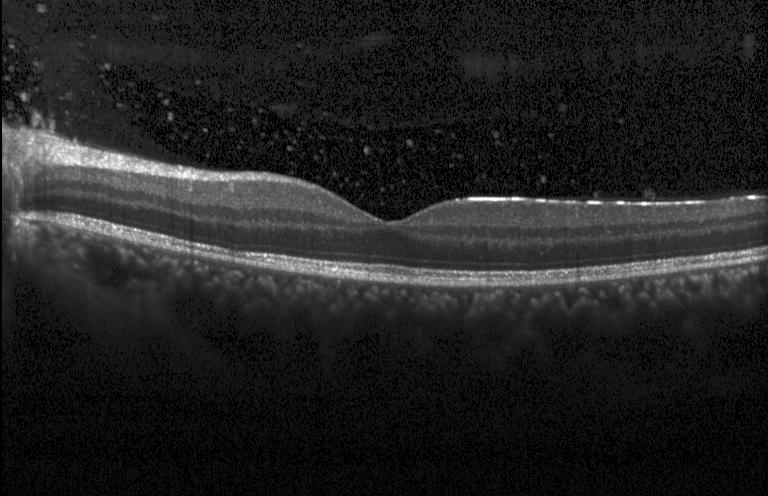
The scan shows neither CNV, DME, nor drusen.